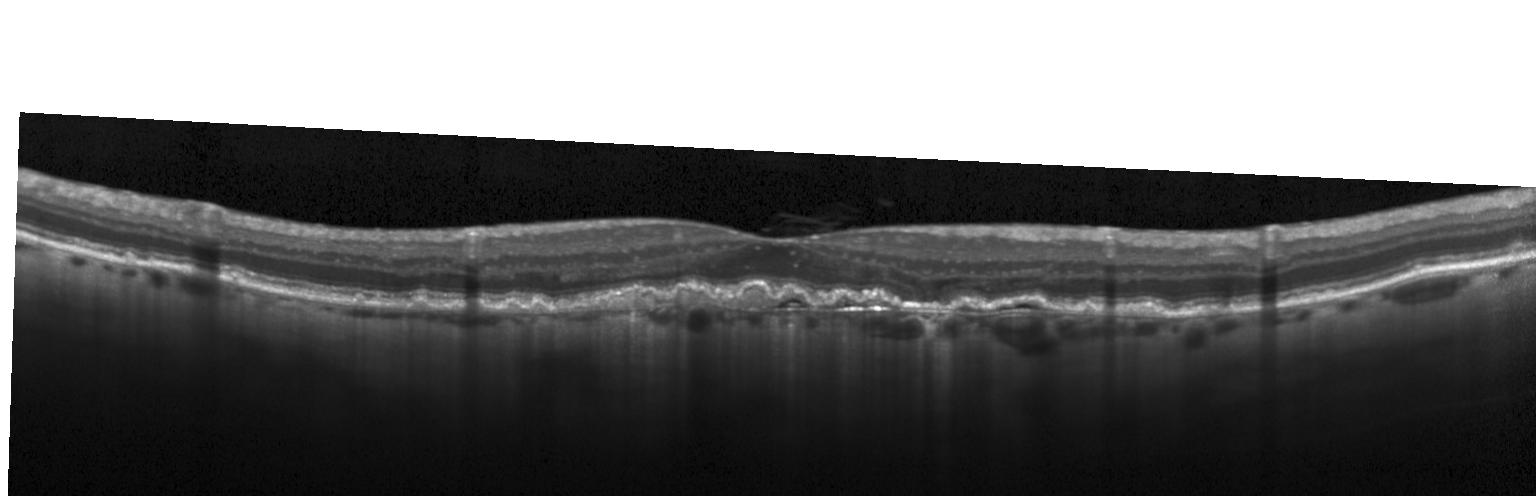
Heidelberg Spectralis OCT system; retinal OCT B-scan
Macular OCT: a choroidal neovascular membrane.